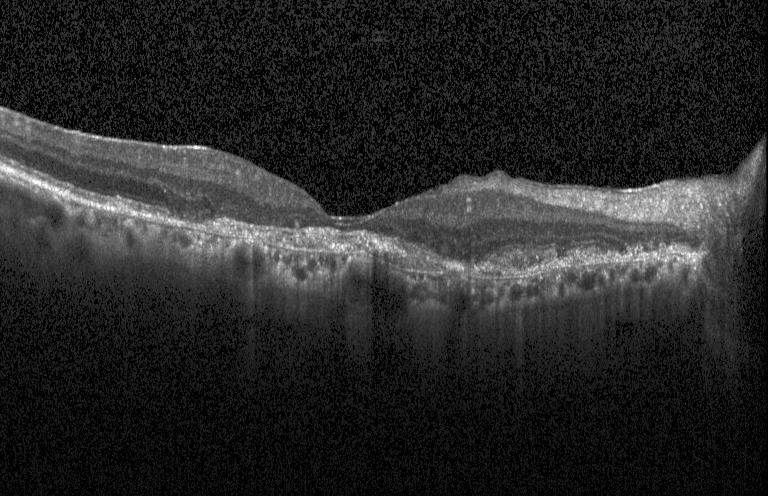

Instrument: Heidelberg Spectralis. Optical coherence tomography scan. Spectral-domain optical coherence tomography. Macular scan — Assessment: CNV.